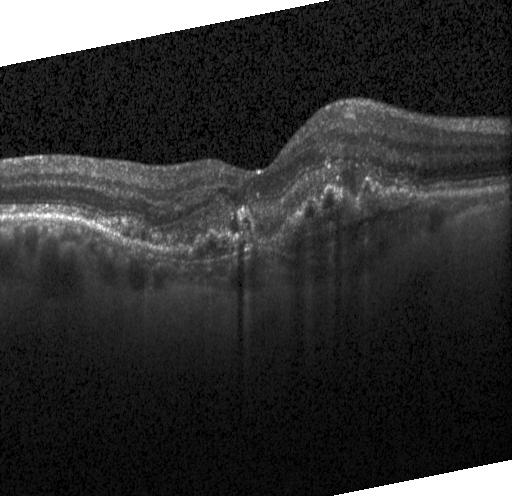

Macular scan · acquired on a Heidelberg Spectralis · OCT B-scan — Macular OCT: a choroidal neovascular membrane.